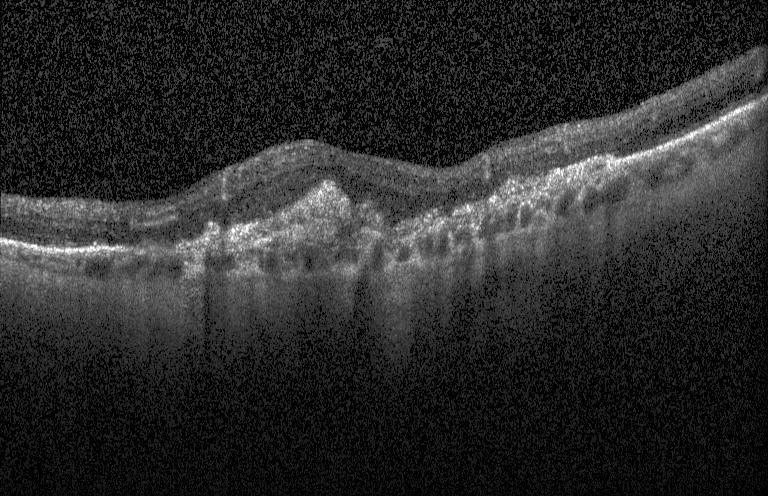
Assessment: a choroidal neovascular membrane.